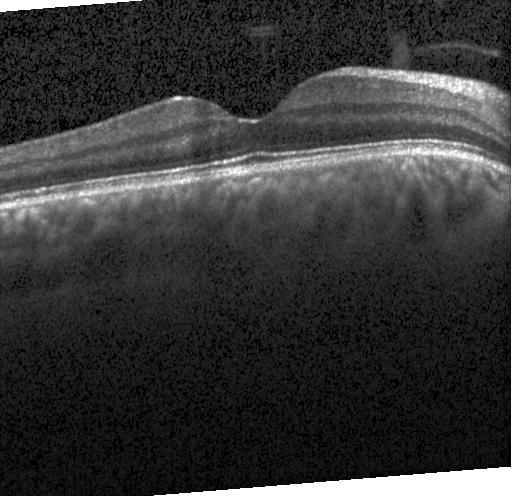

Spectral-domain OCT; fovea-centered; optical coherence tomography B-scan.
Macular OCT: neither CNV, DME, nor drusen.